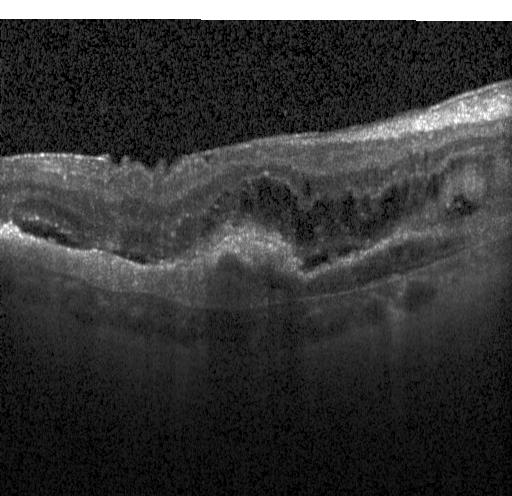

Centered on the fovea; acquired on a Heidelberg Spectralis; spectral-domain optical coherence tomography; OCT line scan. The scan shows a choroidal neovascular membrane.